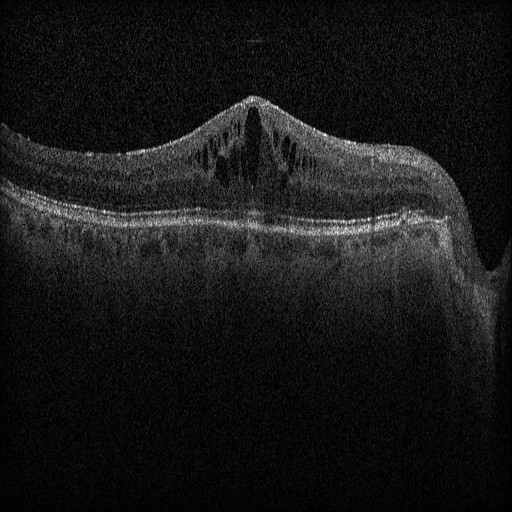
Spectral-domain optical coherence tomography. Fovea-centered. Heidelberg Spectralis OCT system. Retinal OCT cross-section.
The scan shows diabetic macular edema (DME).